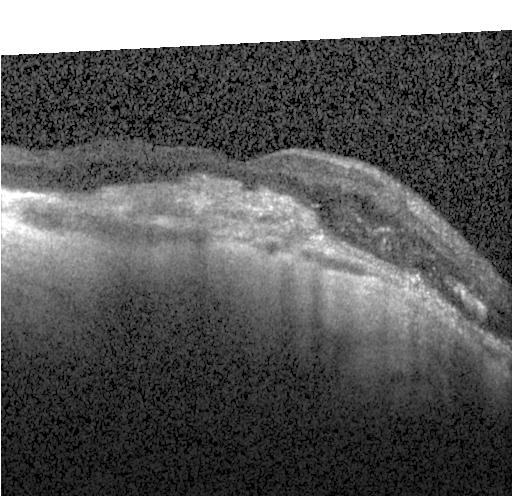 The scan shows a choroidal neovascular membrane.